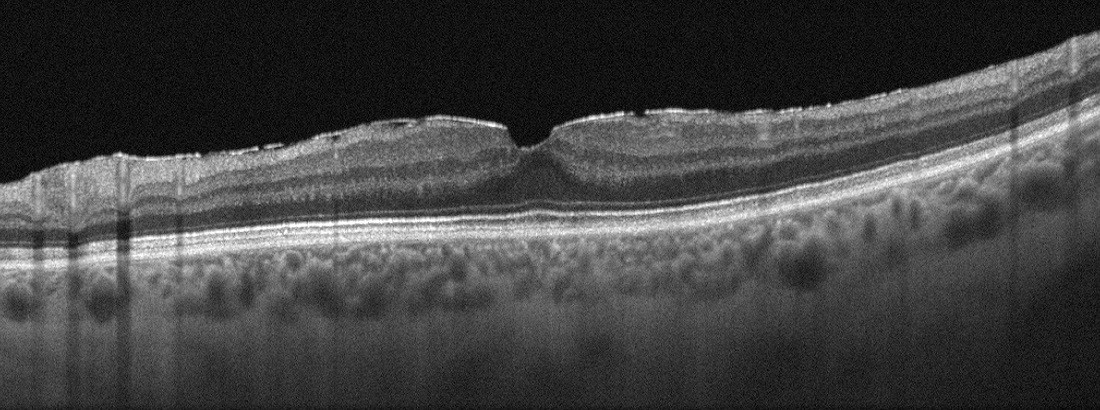

Retinal OCT cross-section. Through the macula. Instrument: Optovue Avanti RTVue XR.
Macular OCT: epiretinal membrane (ERM).